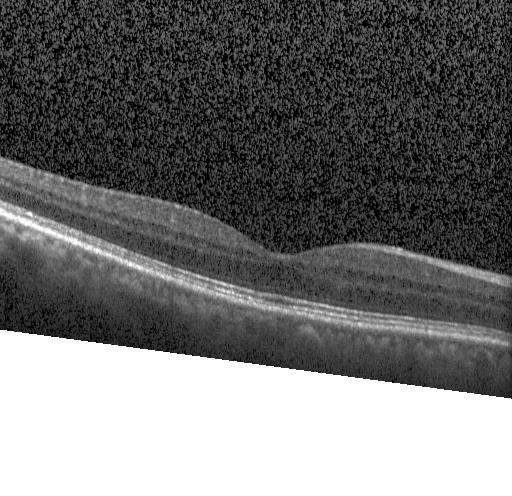 Impression: no evidence of CNV, DME, or drusen.